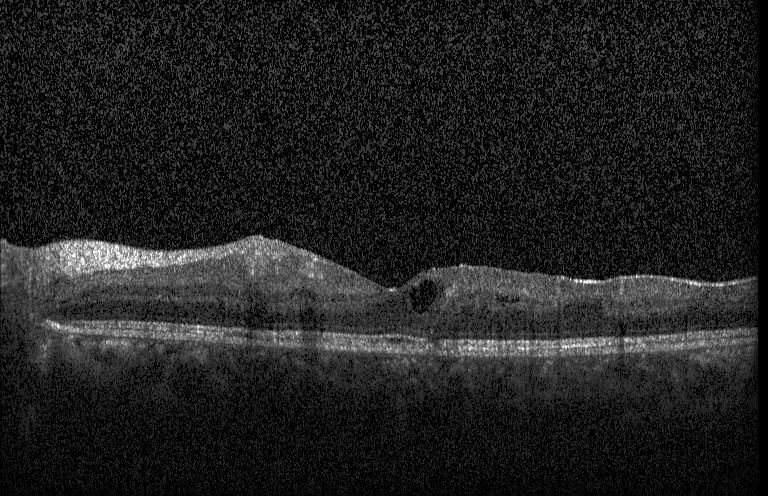 Retinal OCT B-scan.
Impression: DME.